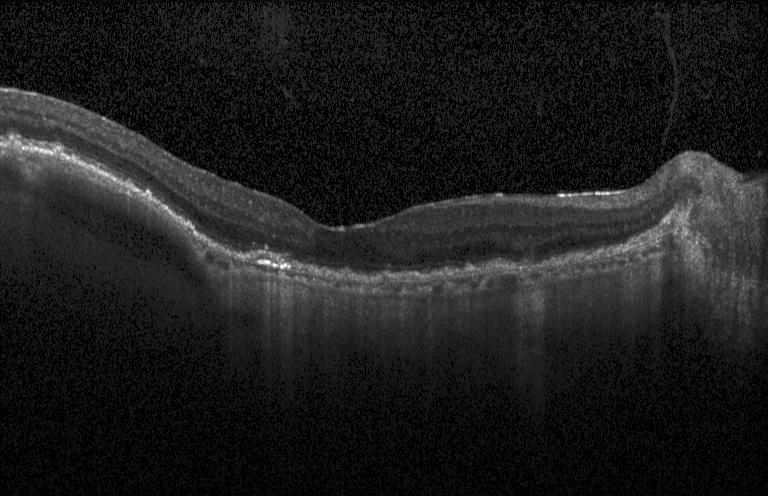

Diagnosis: a choroidal neovascular membrane.